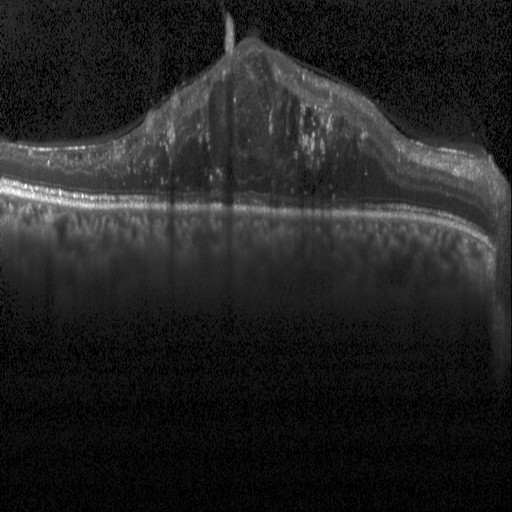

OCT B-scan showing DME.